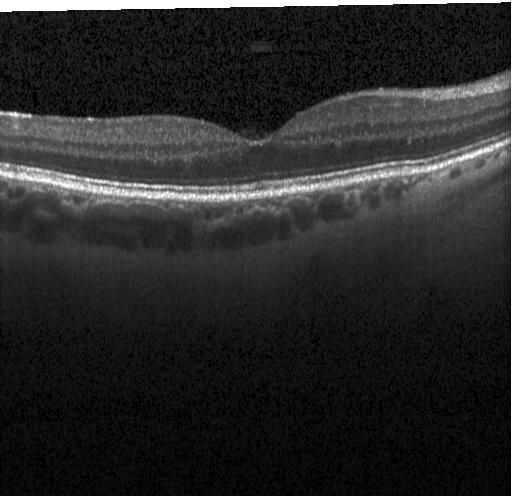 Finding: no CNV, no DME, and no drusen.